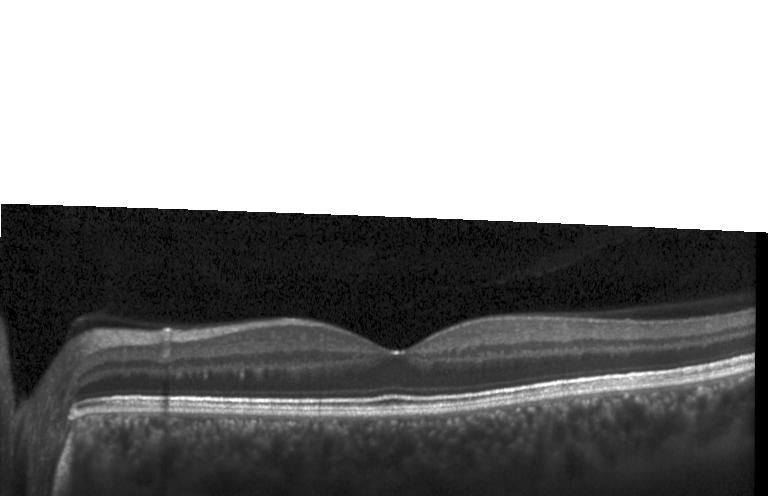 Impression: neither CNV, DME, nor drusen.